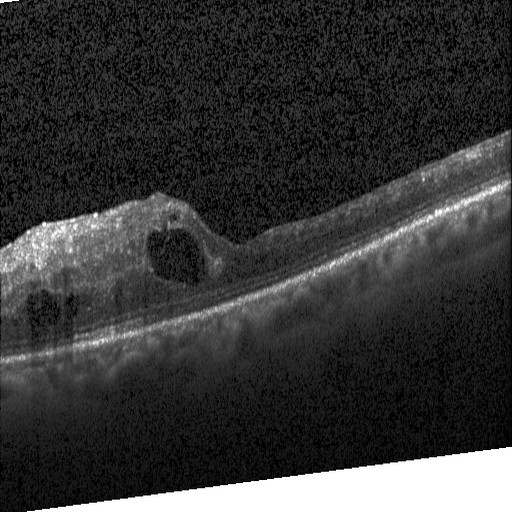
OCT scan showing diabetic macular edema.